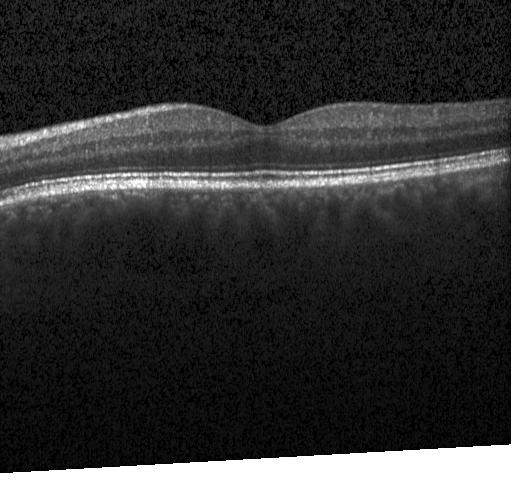 Macular OCT: neither choroidal neovascularization, diabetic macular edema, nor drusen.